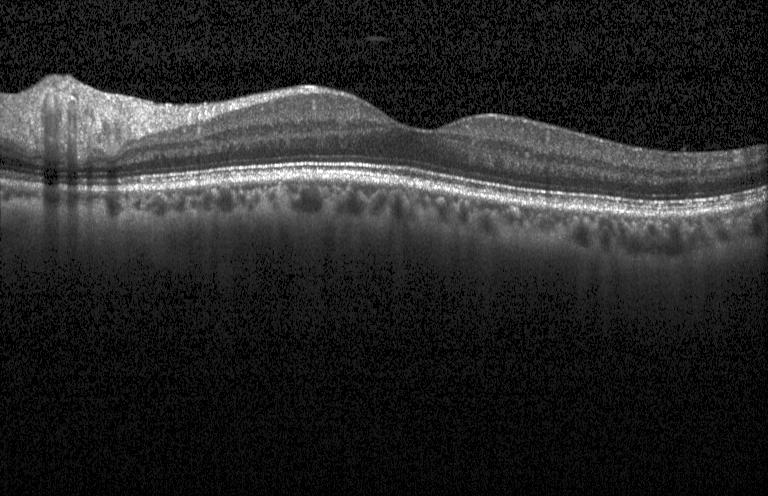

Retinal OCT cross-section showing neither CNV, DME, nor drusen.